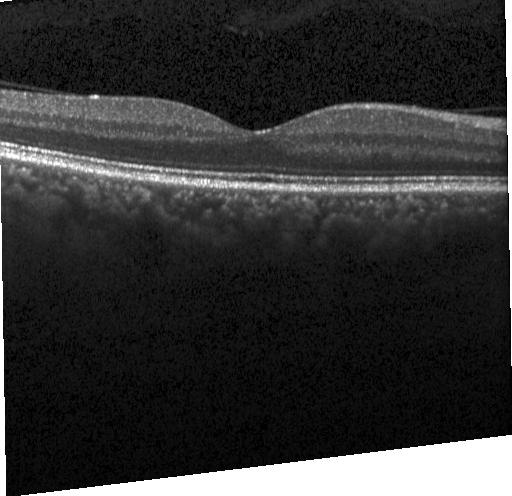
This B-scan demonstrates neither CNV, DME, nor drusen.